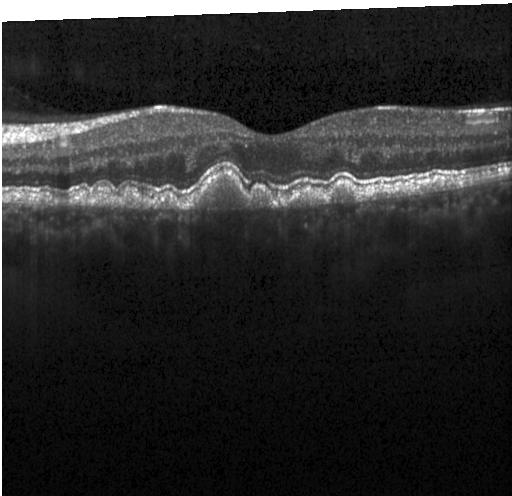
Acquired on a Heidelberg Spectralis; retinal OCT cross-section
Diagnosis: multiple drusen.